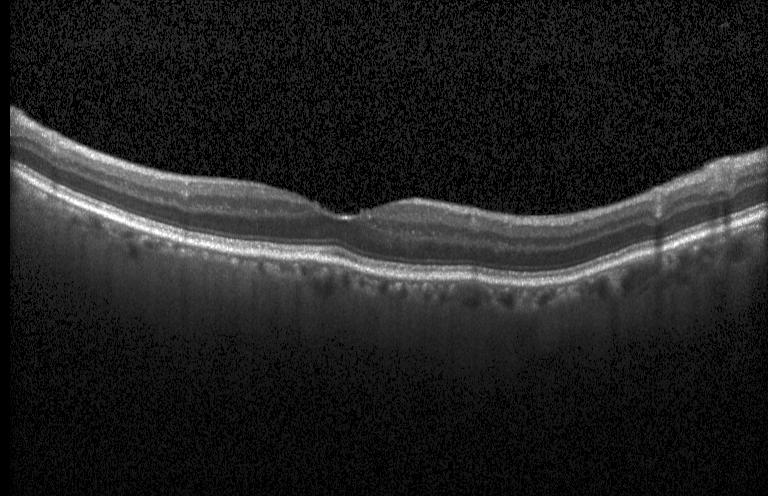

OCT line scan · centered on the fovea · SD-OCT. OCT finding: neither CNV, DME, nor drusen.